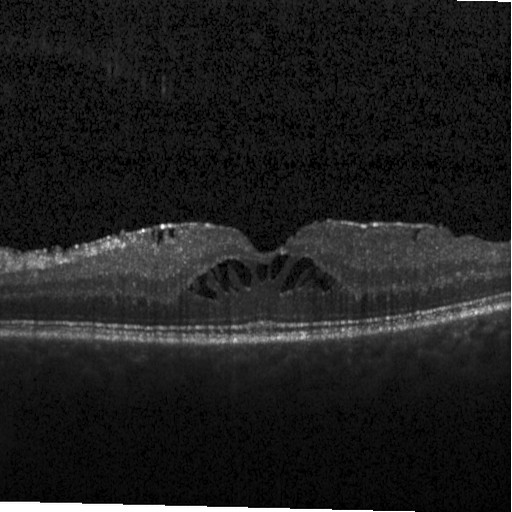 Finding: DME.